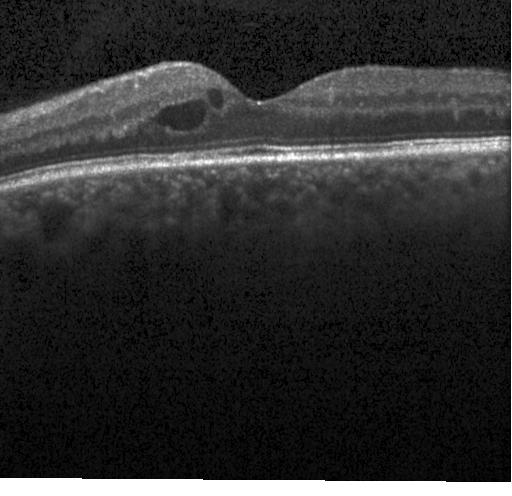 Centered on the fovea. Optical coherence tomography B-scan. SD-OCT.
Diagnosis: diabetic macular edema.